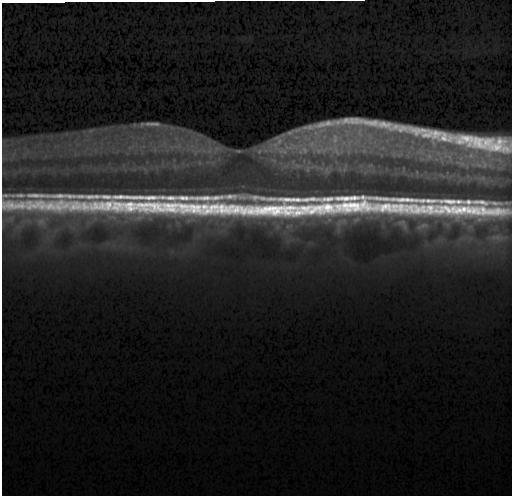

Retinal OCT B-scan. No CNV, no DME, and no drusen.